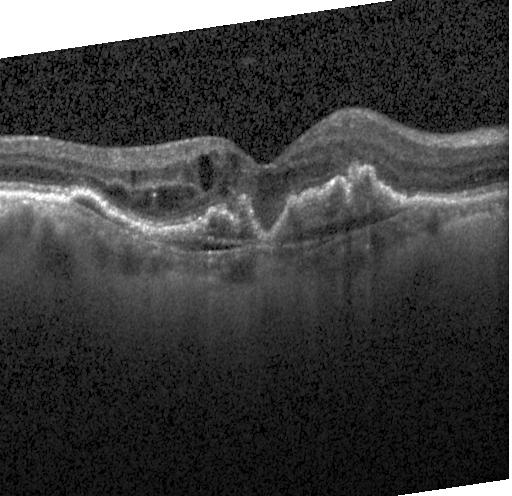
Instrument: Heidelberg Spectralis · retinal OCT cross-section · horizontal scan through the fovea · spectral-domain OCT
Finding: a choroidal neovascular membrane.